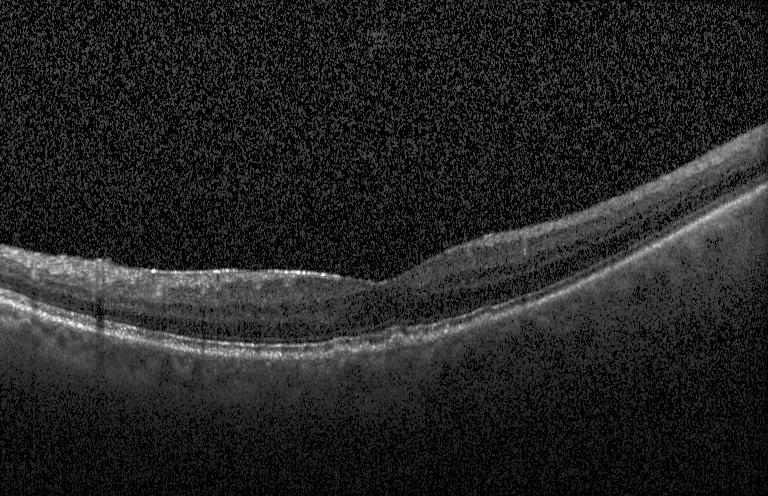
Retinal OCT B-scan, Heidelberg Spectralis, macular scan. Impression: sub-RPE drusenoid deposits.